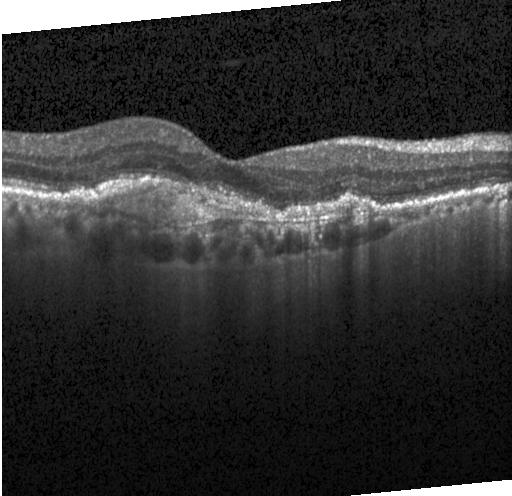 Dx: CNV.